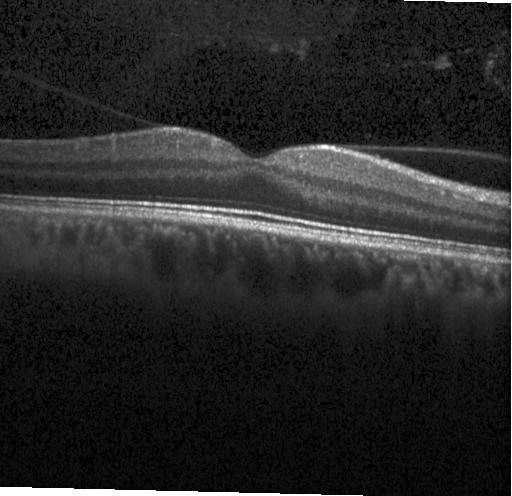

Heidelberg Spectralis. Optical coherence tomography B-scan. Impression: neither choroidal neovascularization, diabetic macular edema, nor drusen.